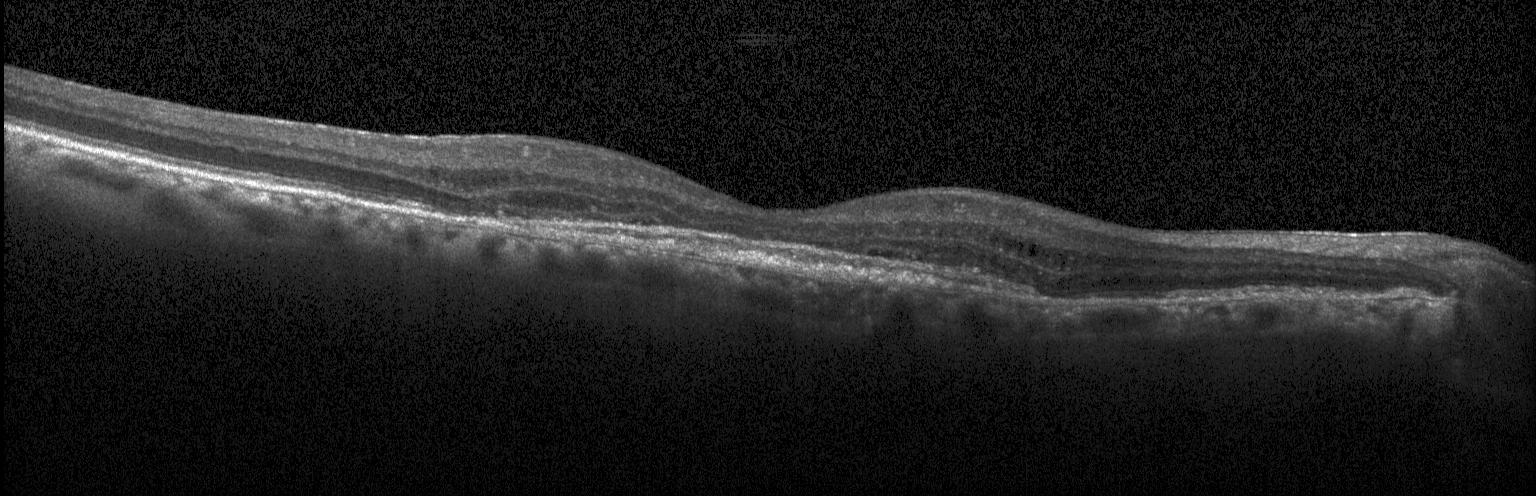

Finding: a choroidal neovascular membrane.